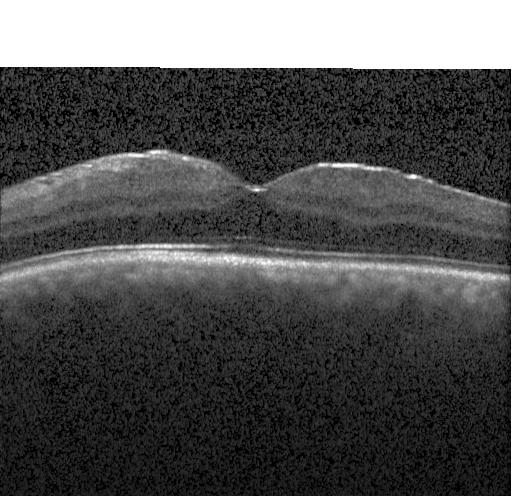
Horizontal scan through the fovea; spectral-domain optical coherence tomography; retinal OCT B-scan; acquired on a Heidelberg Spectralis.
Diagnosis: no choroidal neovascularization, diabetic macular edema, or drusen.